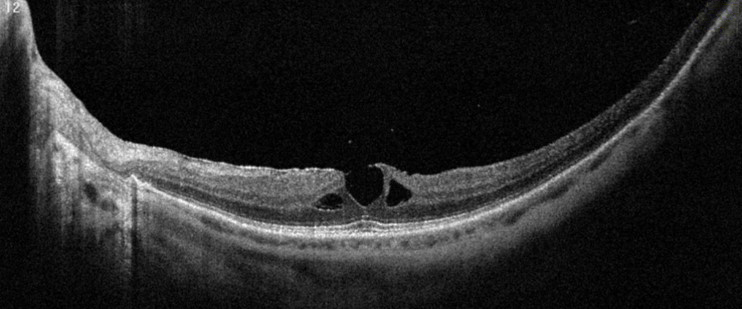 Impression: vitreomacular interface disease (VID).